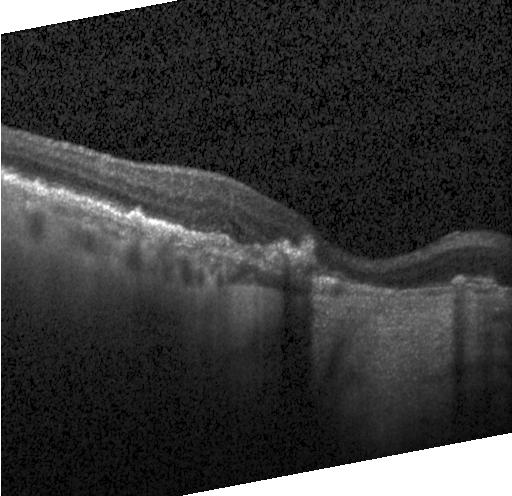

Retinal OCT cross-section showing a choroidal neovascular membrane.